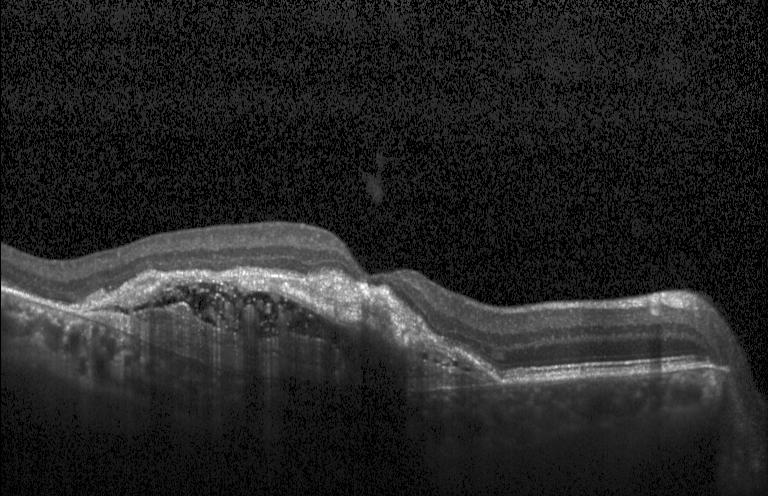 Centered on the fovea, SD-OCT, OCT B-scan — A choroidal neovascular membrane.